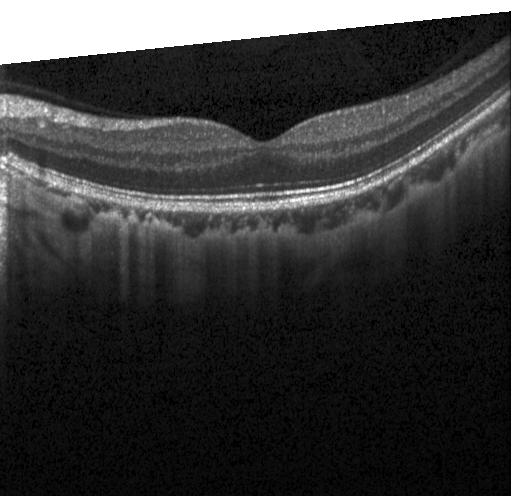 Retinal OCT B-scan. Spectral-domain OCT. Assessment: no choroidal neovascularization, diabetic macular edema, or drusen.